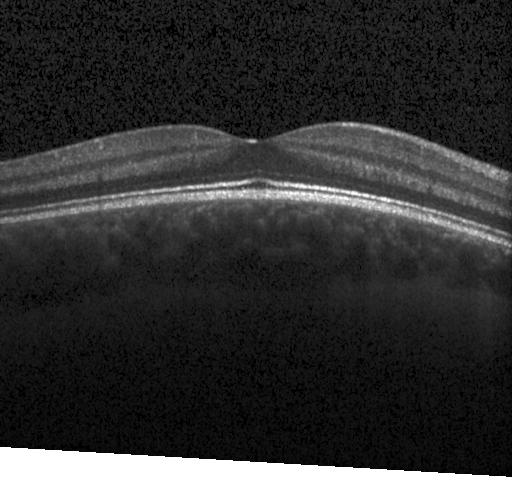

Macular OCT: no choroidal neovascularization, no diabetic macular edema, and no drusen.